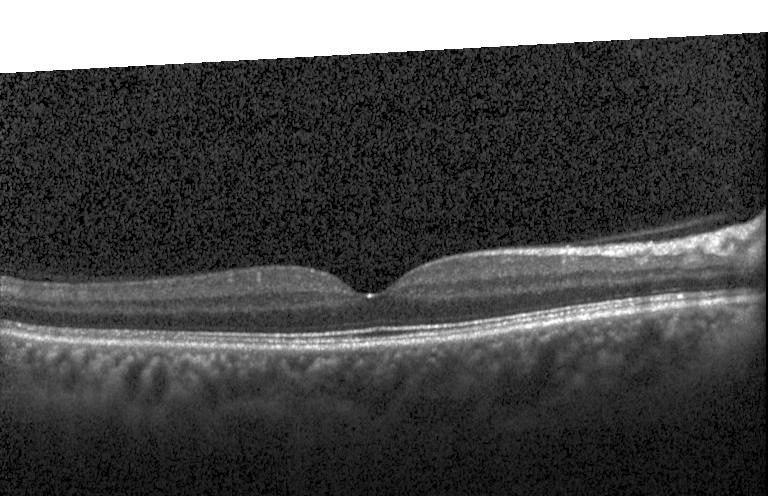

Impression: no evidence of choroidal neovascularization, diabetic macular edema, or drusen.